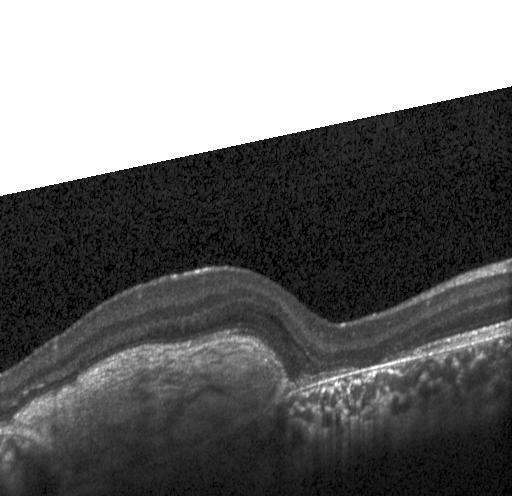

Finding: CNV.